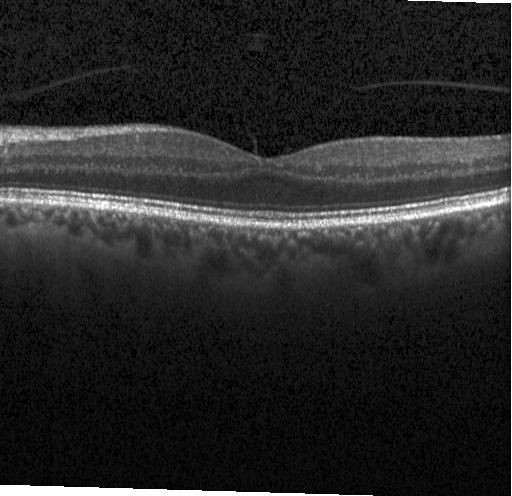 Centered on the fovea; OCT B-scan
Finding: neither choroidal neovascularization, diabetic macular edema, nor drusen.